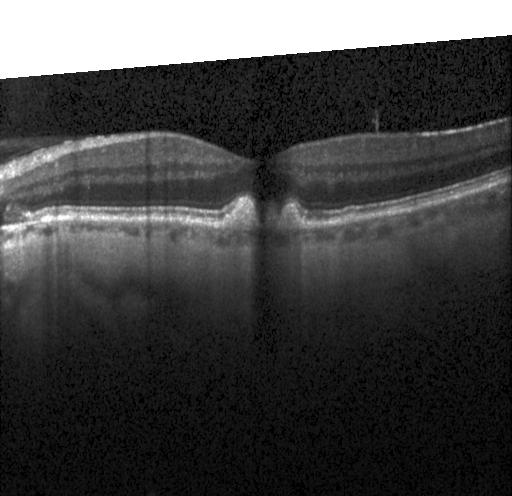

Instrument: Heidelberg Spectralis; retinal OCT cross-section — Assessment: drusen.